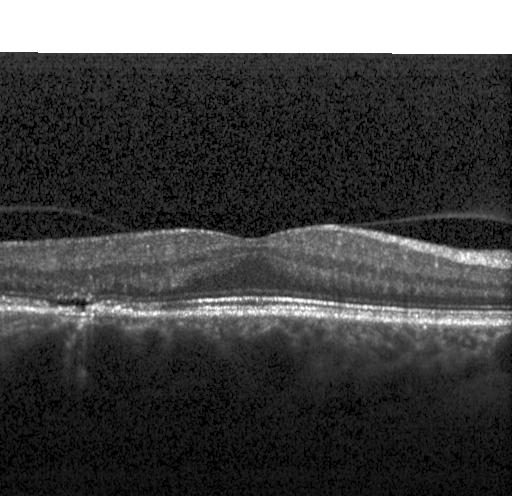

Spectral-domain OCT, retinal OCT cross-section, macular scan. OCT finding: a choroidal neovascular membrane.